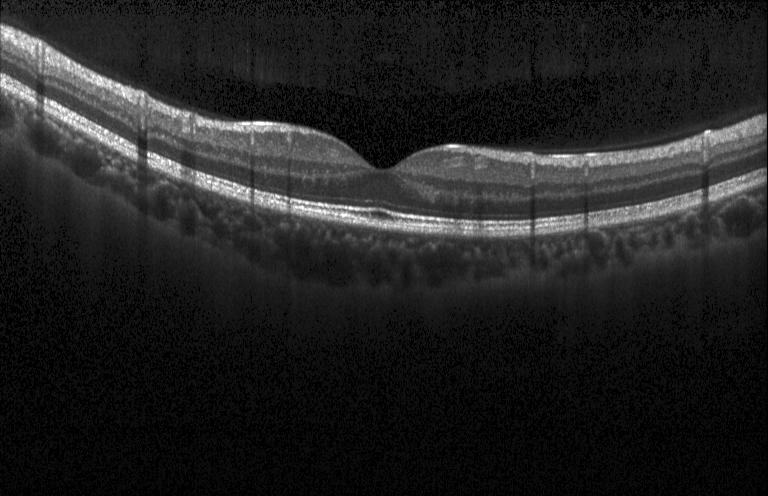

OCT B-scan showing no CNV, DME, or drusen.